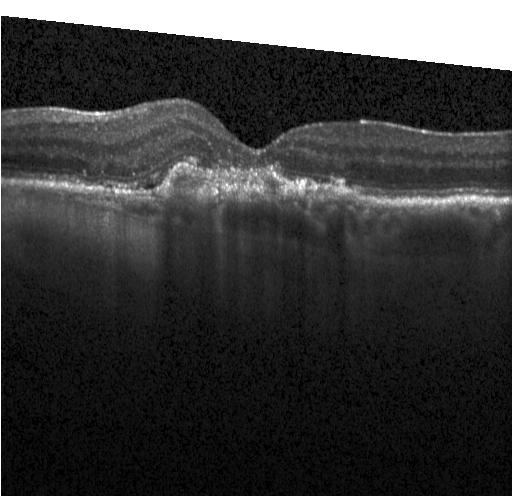
Spectral-domain optical coherence tomography, retinal OCT B-scan, fovea-centered, acquired on a Heidelberg Spectralis. Impression: a choroidal neovascular membrane.